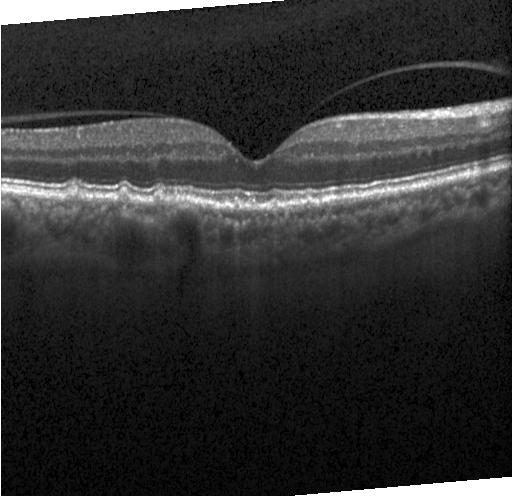

Fovea-centered, retinal OCT B-scan
The scan shows multiple drusen.